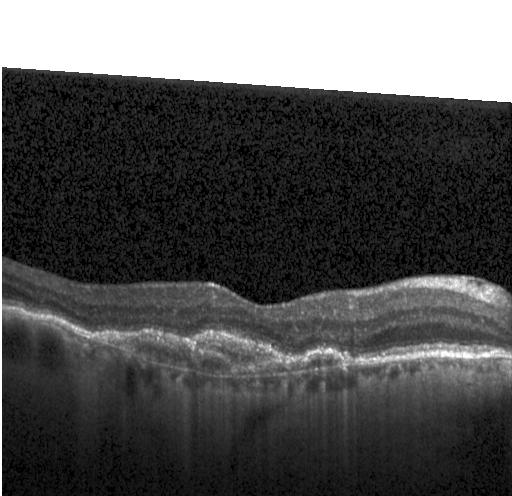

Spectral-domain optical coherence tomography. Optical coherence tomography scan. Diagnosis: a choroidal neovascular membrane.